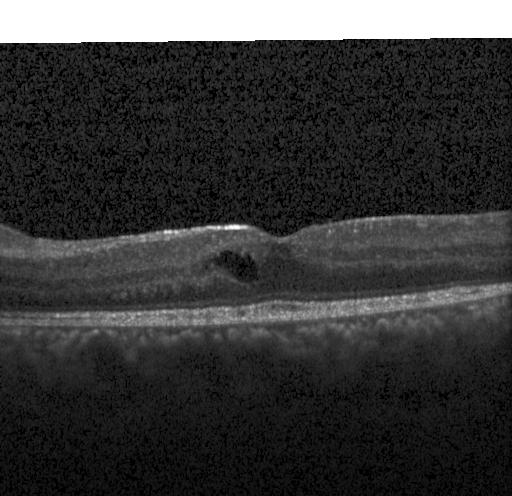 Finding: diabetic macular edema.